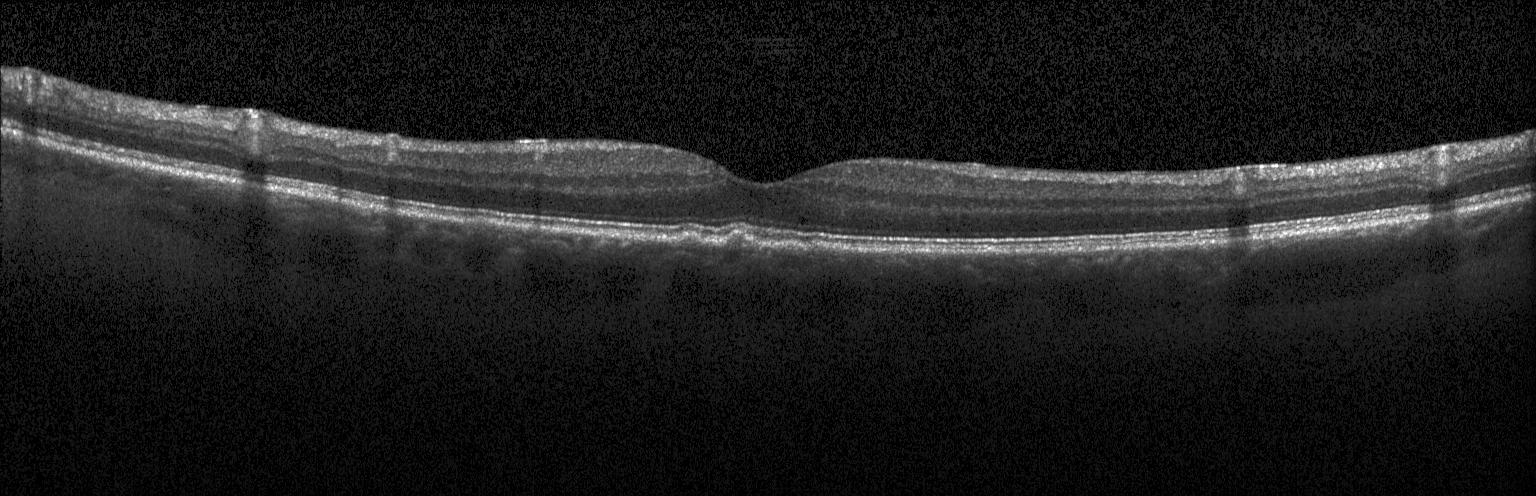 Impression: sub-RPE drusenoid deposits.